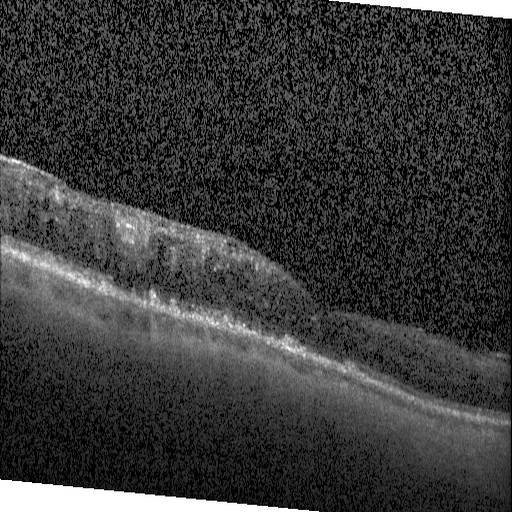
Impression: diabetic macular edema (DME).